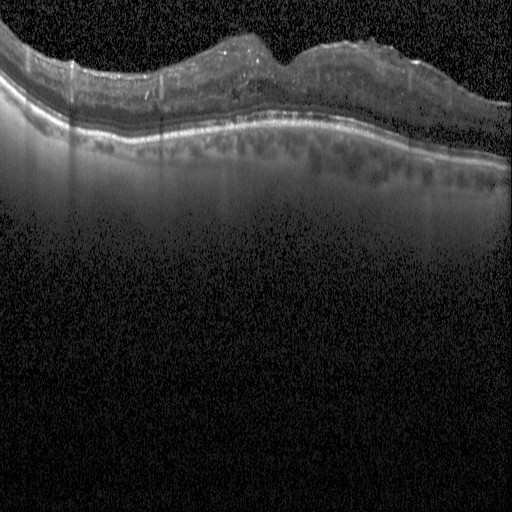 Instrument: Heidelberg Spectralis; spectral-domain optical coherence tomography; optical coherence tomography scan; macular scan
The scan shows diabetic macular edema.